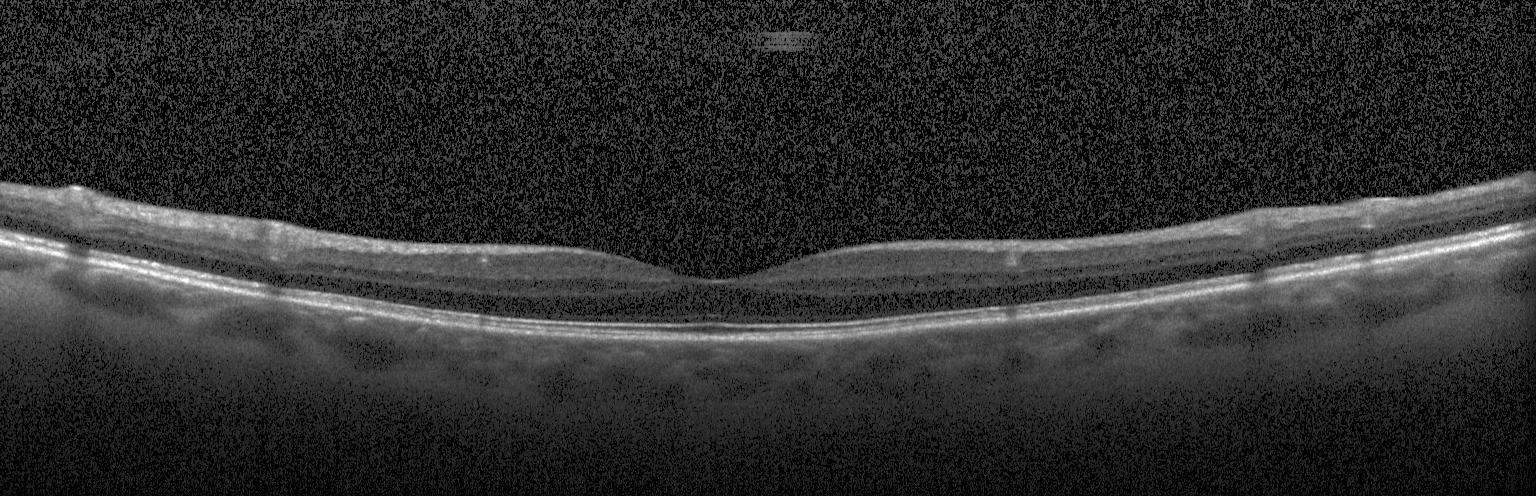

Finding: no evidence of choroidal neovascularization, diabetic macular edema, or drusen.